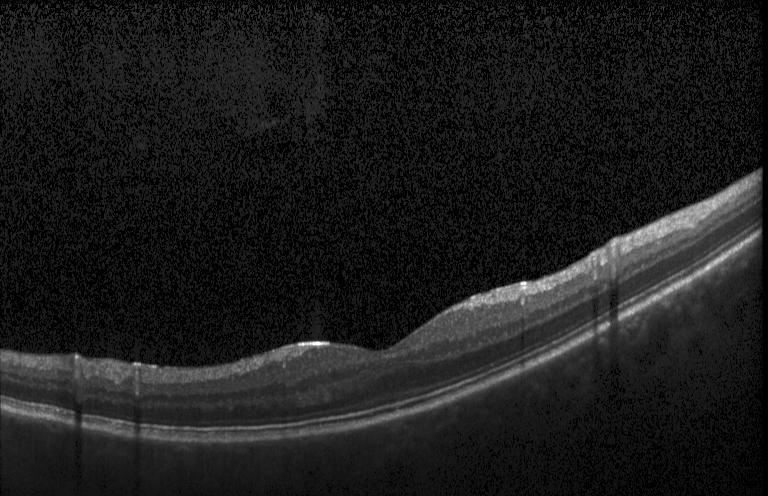

Impression: no evidence of choroidal neovascularization, diabetic macular edema, or drusen.